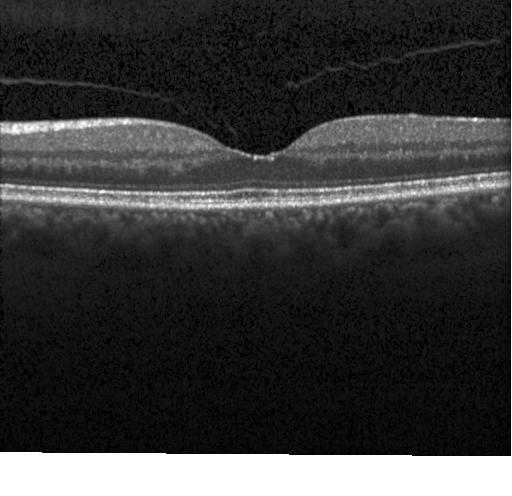
Optical coherence tomography scan · horizontal scan through the fovea · acquired on a Heidelberg Spectralis. Dx: no evidence of CNV, DME, or drusen.